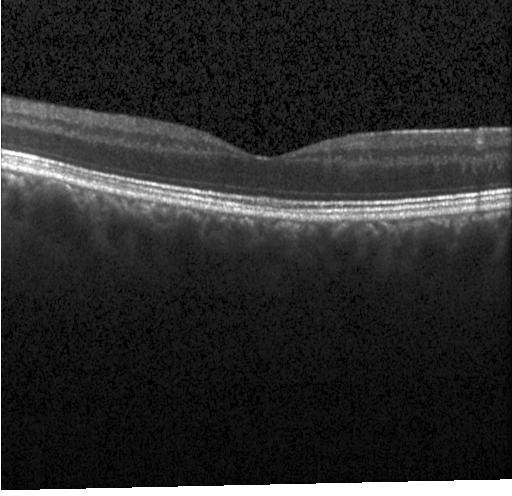 Acquired on a Heidelberg Spectralis. SD-OCT. OCT line scan. Macular scan. This B-scan demonstrates no evidence of choroidal neovascularization, diabetic macular edema, or drusen.